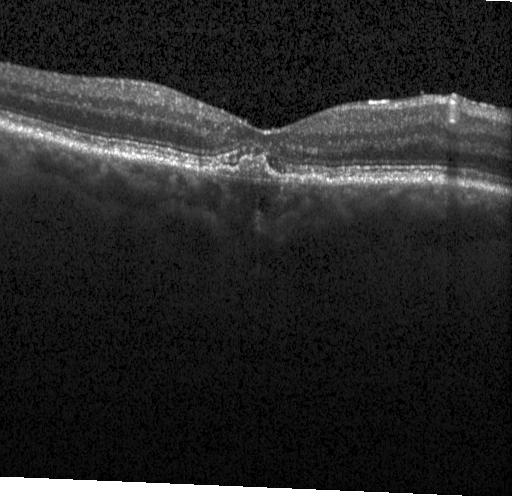
Optical coherence tomography B-scan
Macular OCT: choroidal neovascularization.